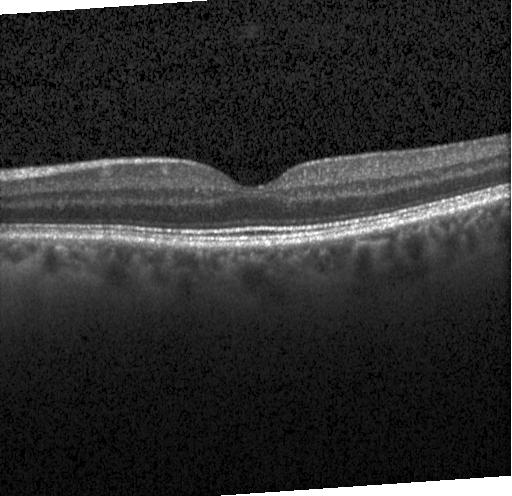
This B-scan demonstrates no evidence of CNV, DME, or drusen.